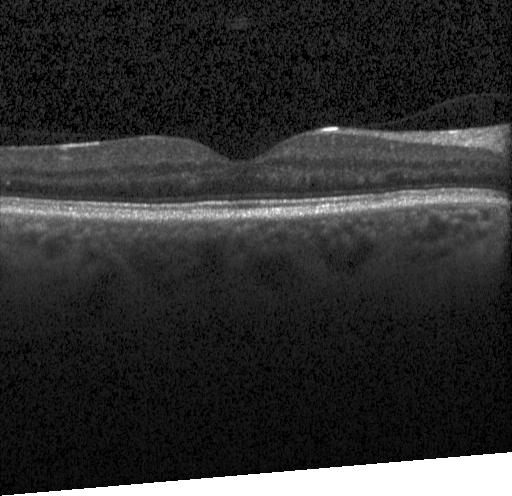
OCT B-scan. Assessment: no choroidal neovascularization, diabetic macular edema, or drusen.